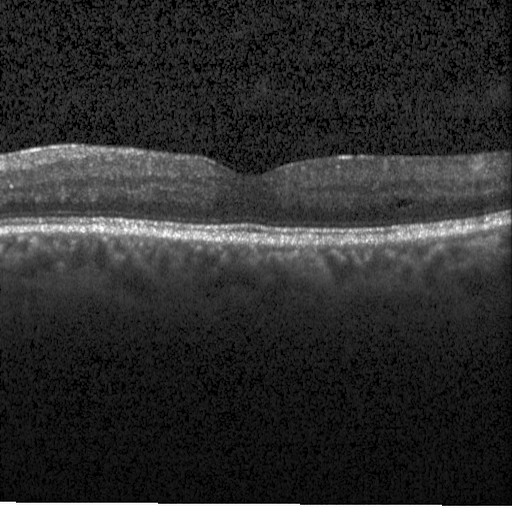
Macular scan; OCT line scan; spectral-domain OCT — Impression: diabetic macular edema (DME).